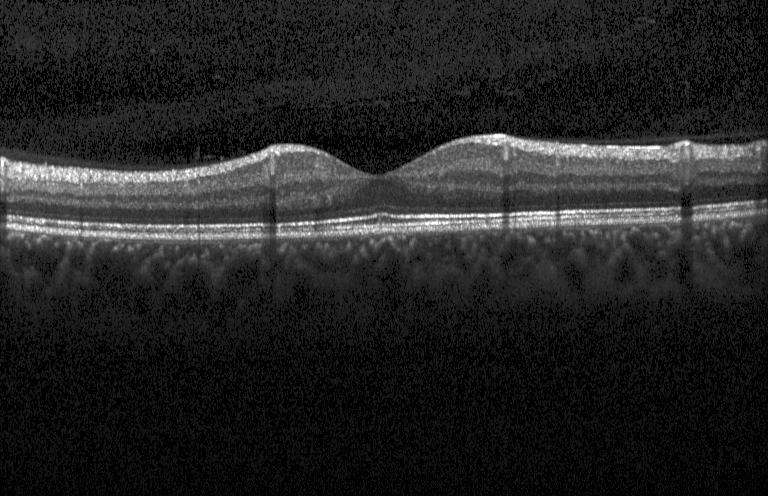
Dx: no choroidal neovascularization, diabetic macular edema, or drusen.